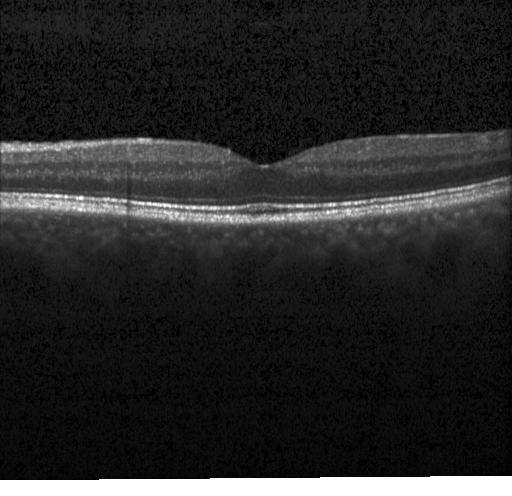 Diagnosis: no choroidal neovascularization, diabetic macular edema, or drusen.